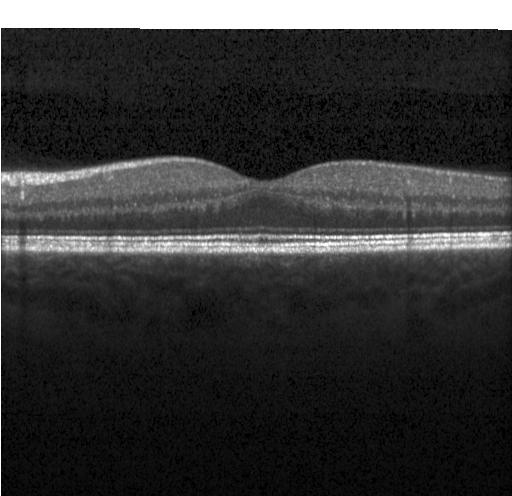

Diagnosis: no choroidal neovascularization, no diabetic macular edema, and no drusen.